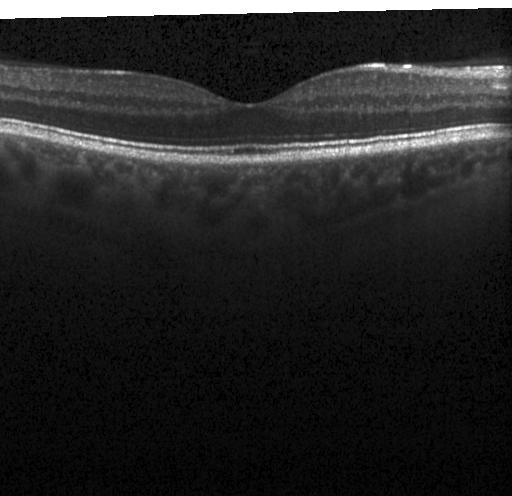

This B-scan demonstrates neither choroidal neovascularization, diabetic macular edema, nor drusen.